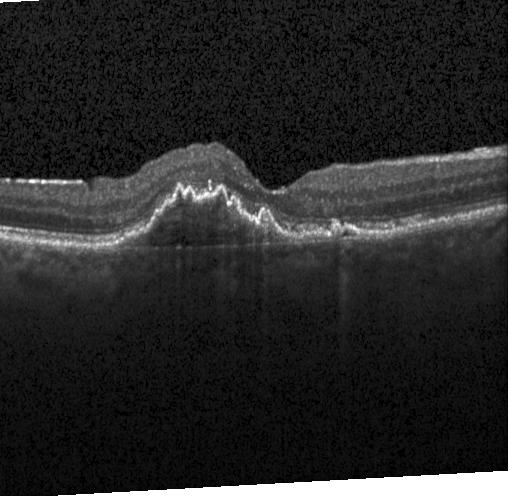 Macular OCT: choroidal neovascularization.